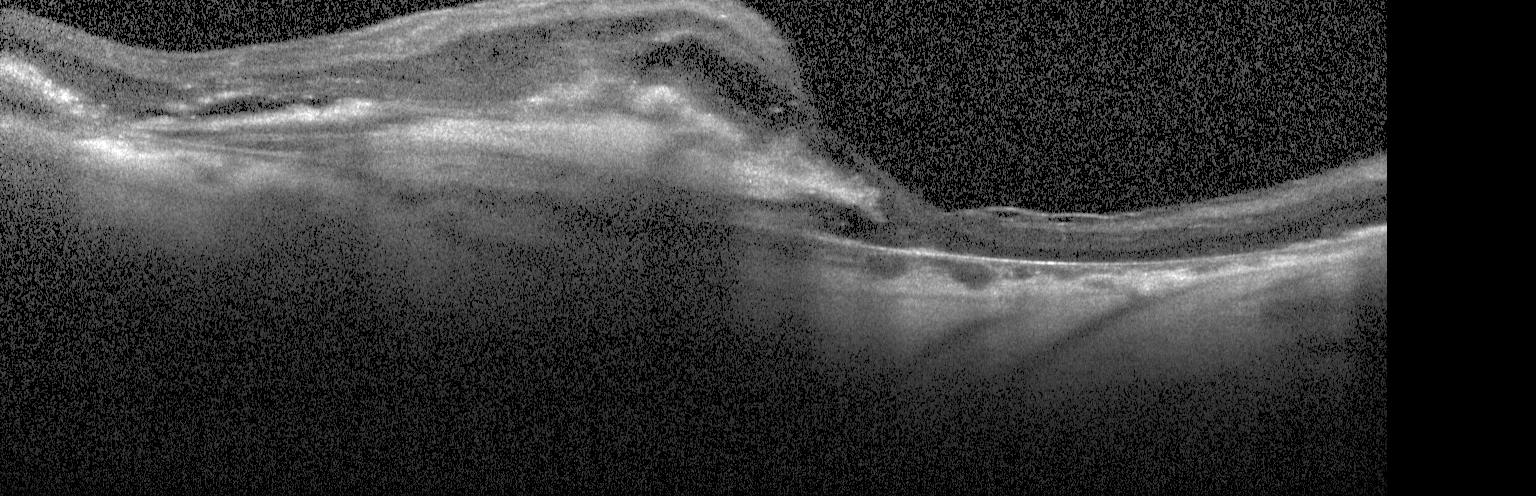

Through the macula. Acquired on a Heidelberg Spectralis. Retinal OCT B-scan. Spectral-domain optical coherence tomography — Choroidal neovascularization (CNV).